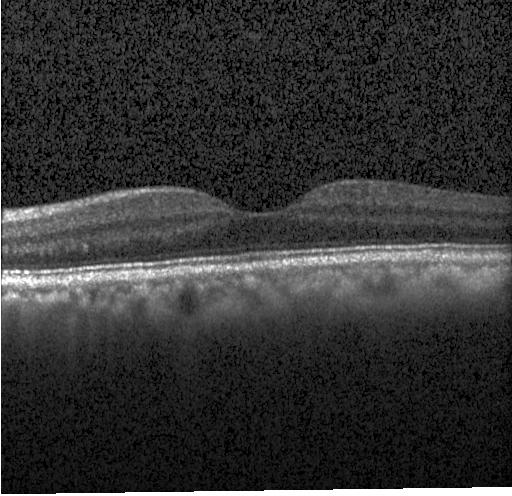

Optical coherence tomography scan. Diagnosis: no choroidal neovascularization, no diabetic macular edema, and no drusen.